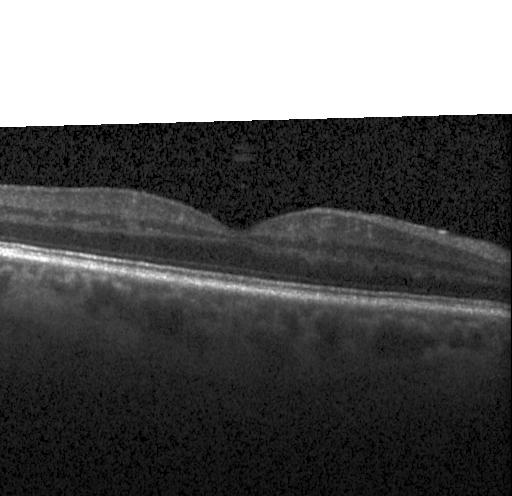

SD-OCT; through the macula; optical coherence tomography B-scan
Macular OCT: neither choroidal neovascularization, diabetic macular edema, nor drusen.